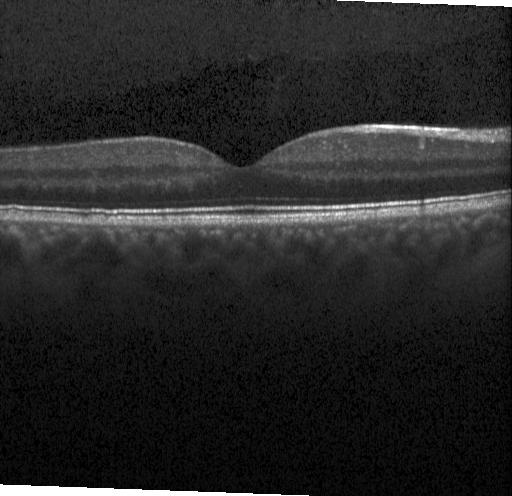 Assessment: neither choroidal neovascularization, diabetic macular edema, nor drusen.